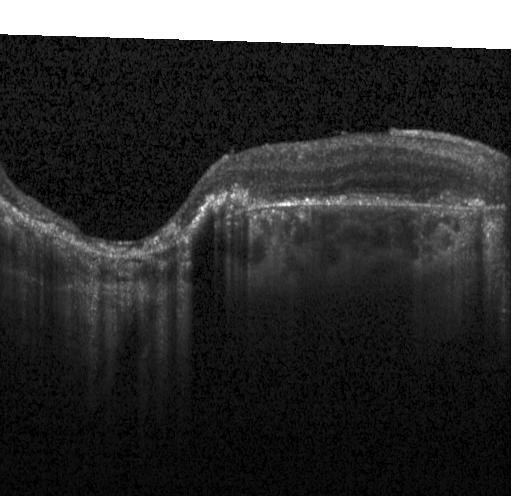
Retinal OCT B-scan. Instrument: Heidelberg Spectralis
The scan shows CNV.